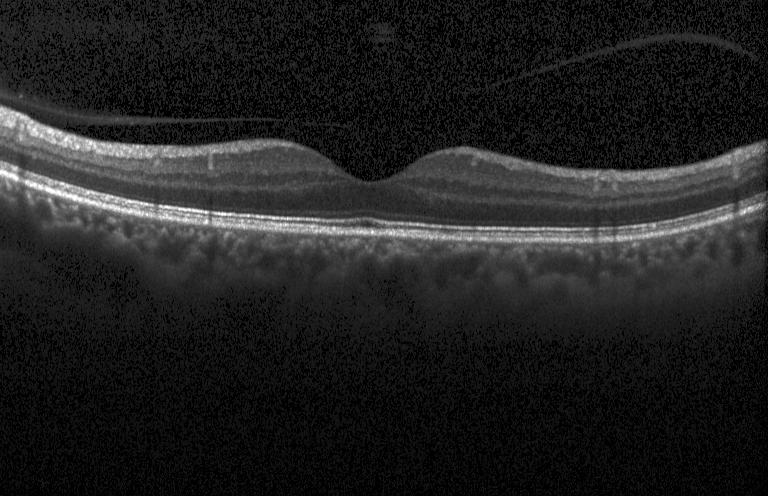 OCT line scan · macular scan. Impression: no choroidal neovascularization, no diabetic macular edema, and no drusen.